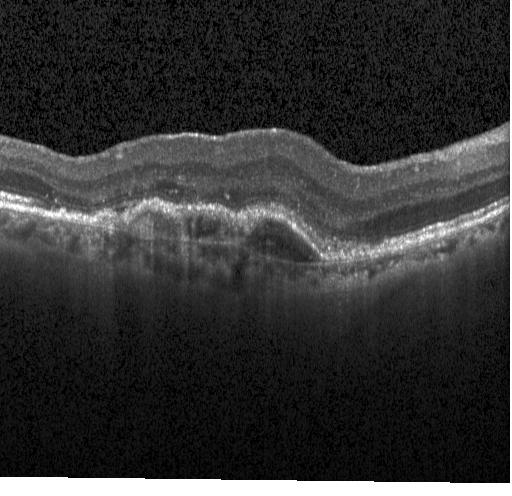
Retinal OCT cross-section. This B-scan demonstrates choroidal neovascularization.